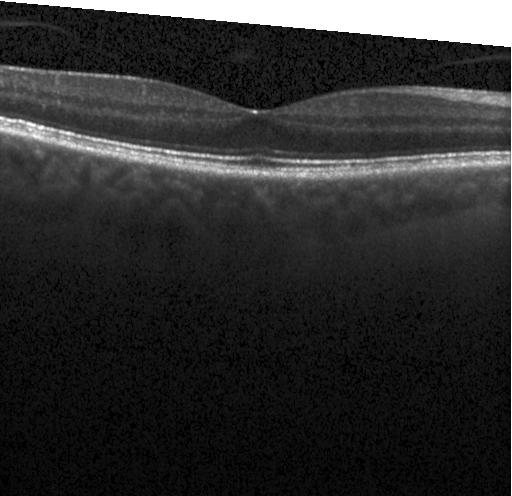 Fovea-centered. Spectral-domain OCT. Instrument: Heidelberg Spectralis. Optical coherence tomography scan — The scan shows neither choroidal neovascularization, diabetic macular edema, nor drusen.